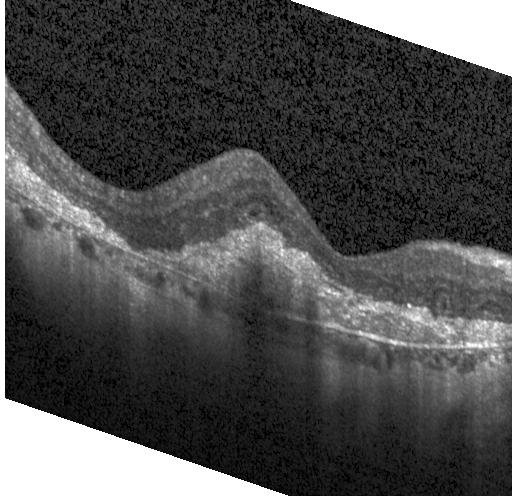
Through the macula; retinal OCT B-scan; Heidelberg Spectralis OCT system
This B-scan demonstrates choroidal neovascularization.